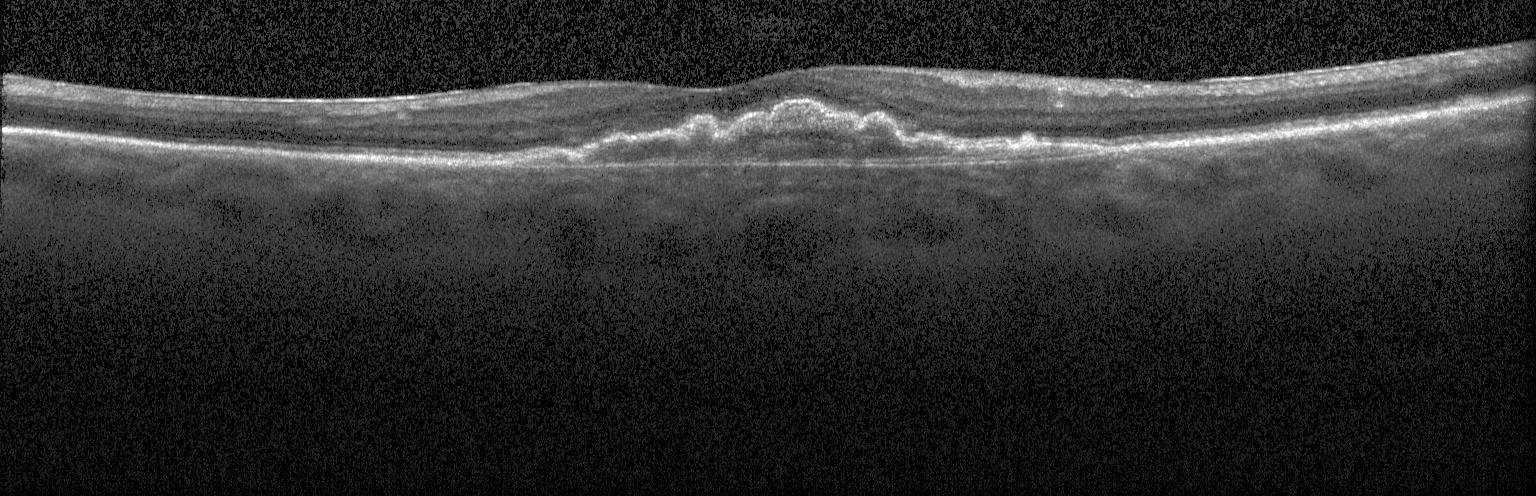 SD-OCT, optical coherence tomography B-scan, fovea-centered — Diagnosis: CNV.